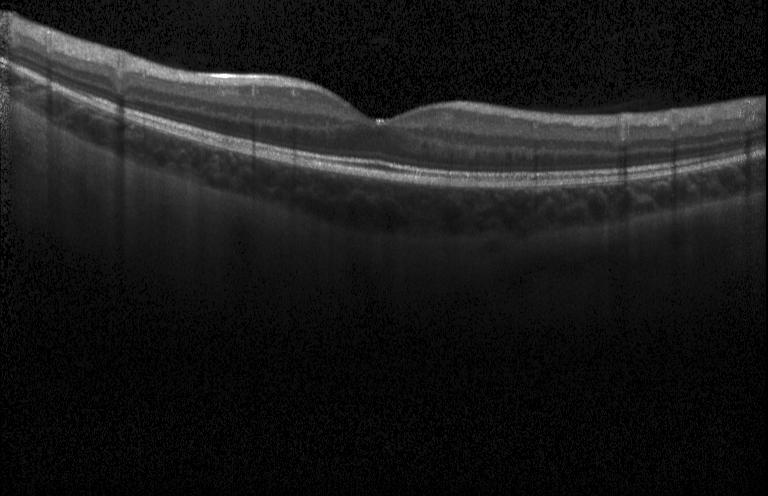

Horizontal scan through the fovea · optical coherence tomography scan.
No evidence of CNV, DME, or drusen.